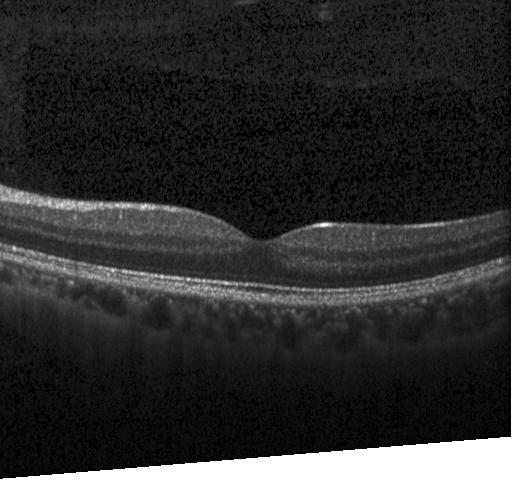

This B-scan demonstrates neither CNV, DME, nor drusen.